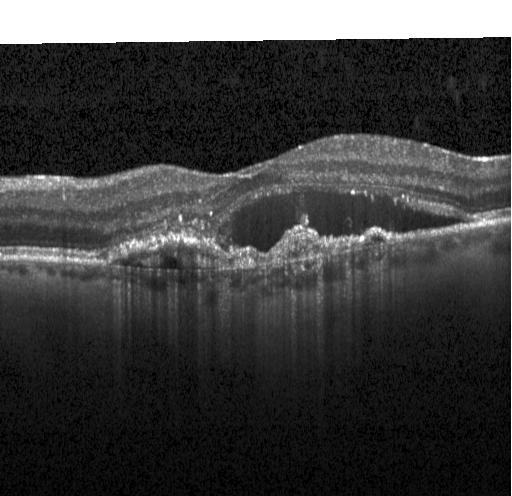

OCT B-scan showing choroidal neovascularization.